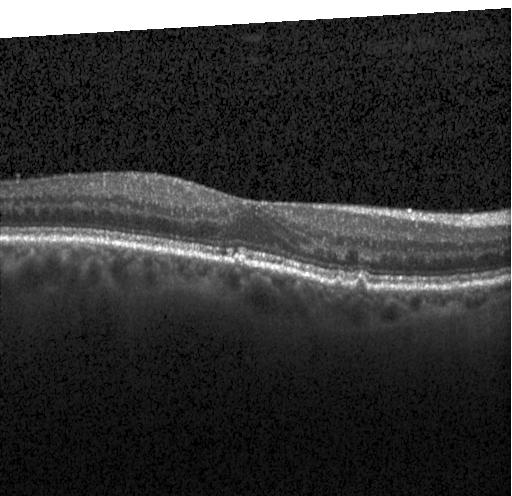 Impression: sub-RPE drusenoid deposits.